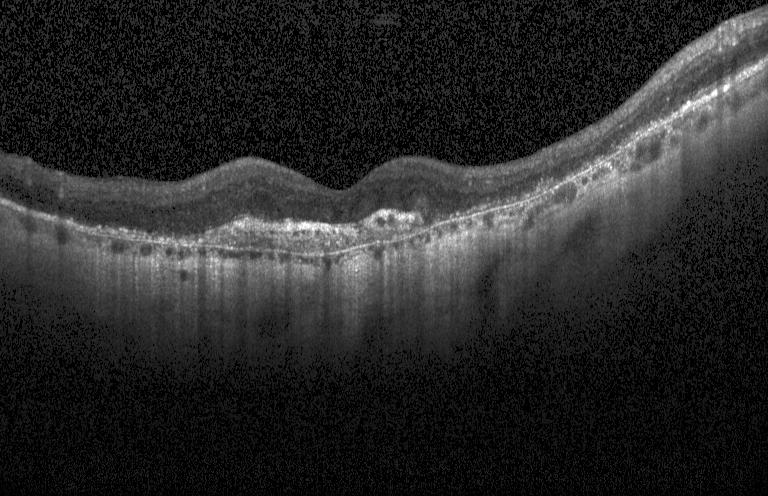 Optical coherence tomography B-scan
Diagnosis: CNV.